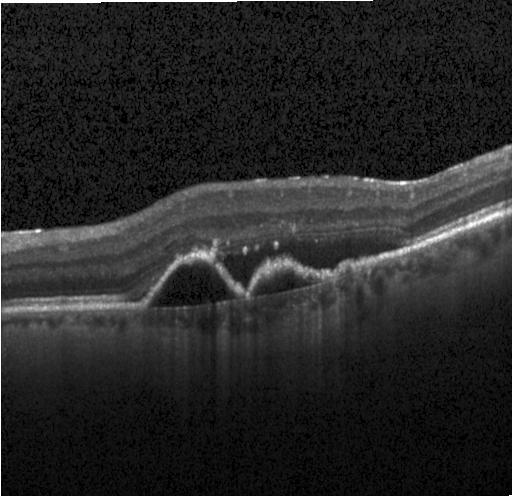 OCT B-scan; through the macula; spectral-domain OCT; instrument: Heidelberg Spectralis. Finding: a choroidal neovascular membrane.